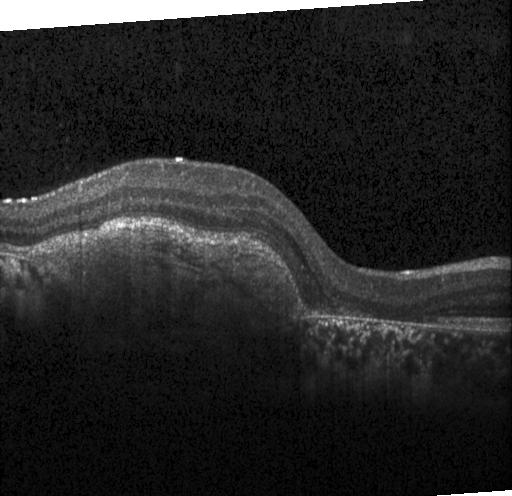

Impression: choroidal neovascularization (CNV).